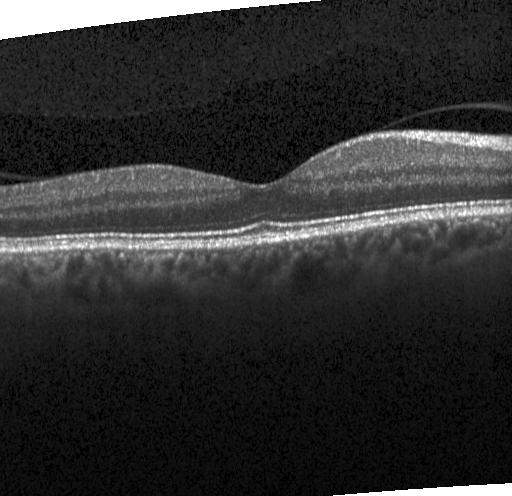
Spectral-domain optical coherence tomography; retinal OCT cross-section; Heidelberg Spectralis — Finding: no CNV, DME, or drusen.